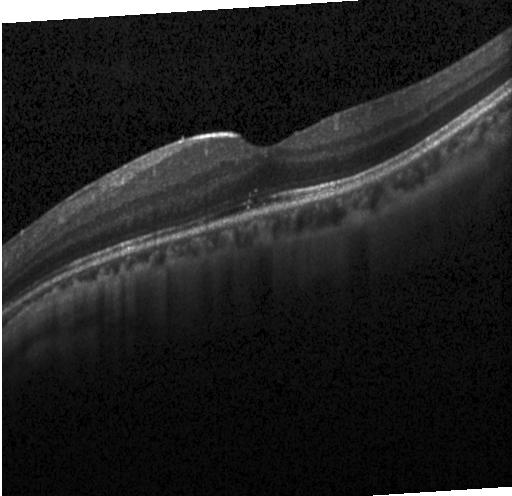
Retinal OCT B-scan. Heidelberg Spectralis OCT system. Macular OCT: no choroidal neovascularization, diabetic macular edema, or drusen.